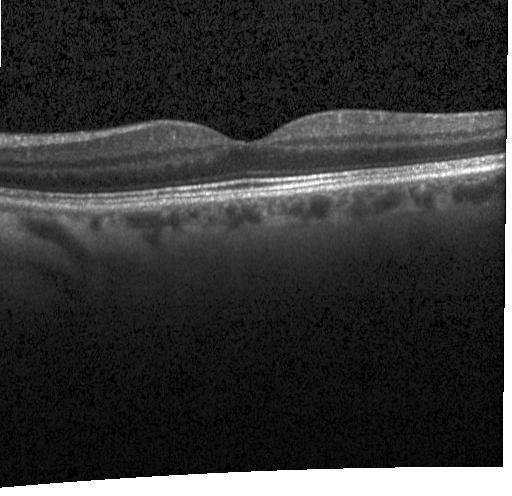
OCT scan showing no choroidal neovascularization, no diabetic macular edema, and no drusen.